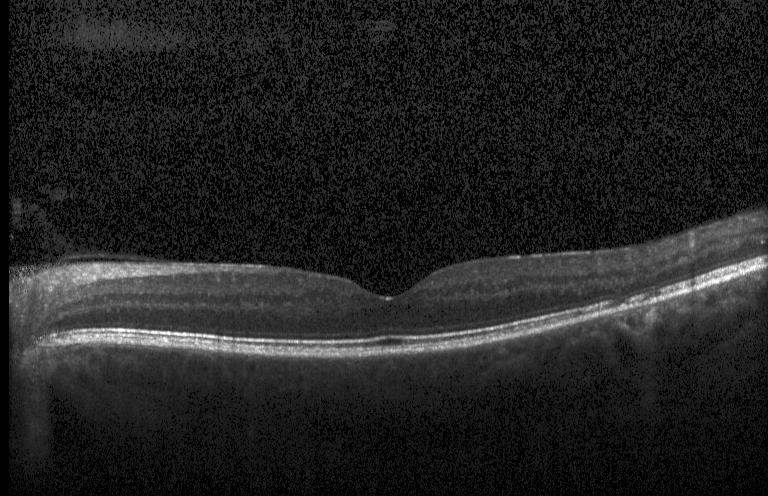
Optical coherence tomography B-scan — Diagnosis: no choroidal neovascularization, diabetic macular edema, or drusen.